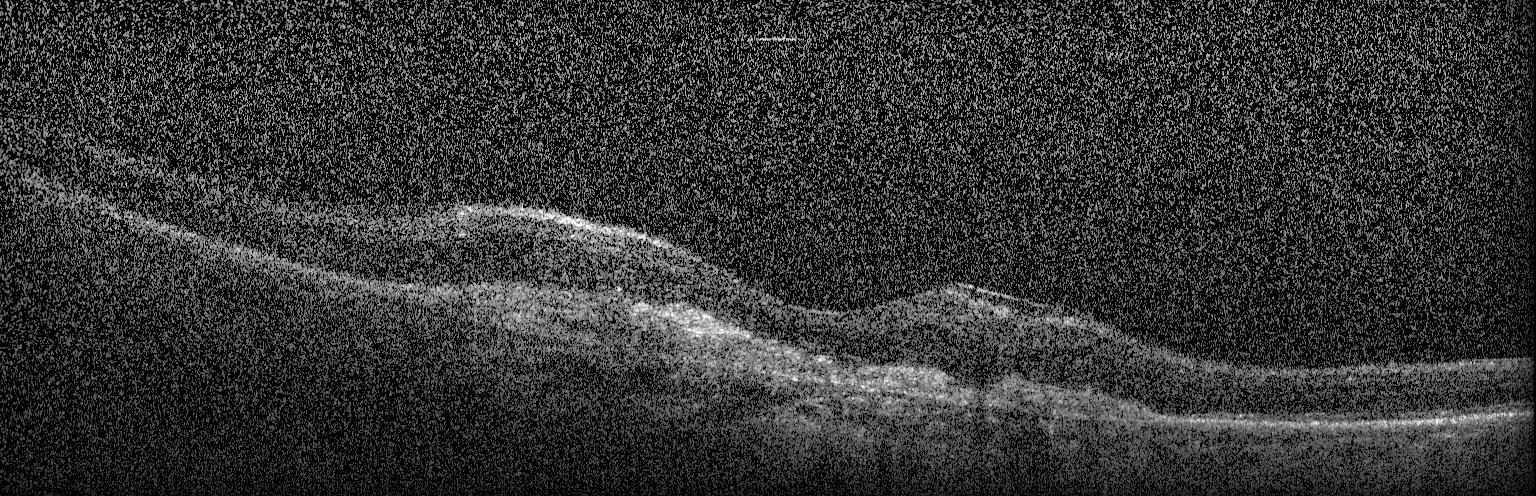
OCT B-scan. OCT finding: a choroidal neovascular membrane.